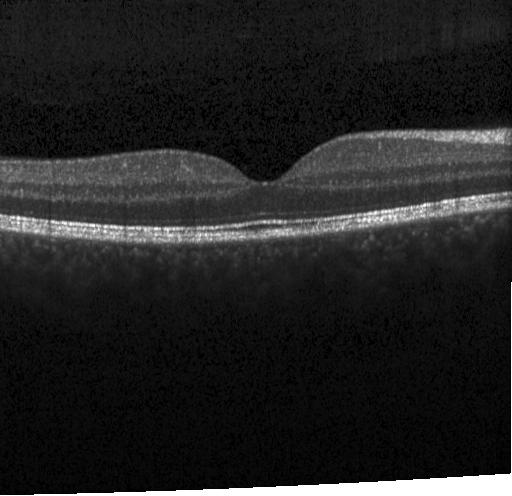

Optical coherence tomography B-scan — Assessment: no choroidal neovascularization, diabetic macular edema, or drusen.